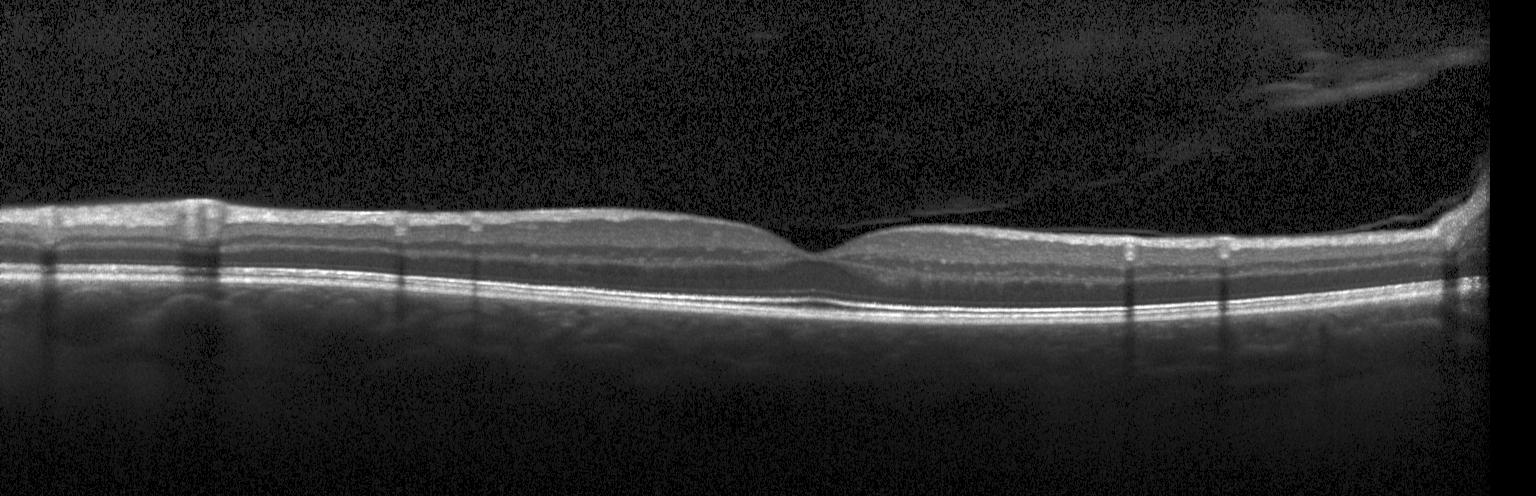
Retinal OCT cross-section showing no evidence of choroidal neovascularization, diabetic macular edema, or drusen.